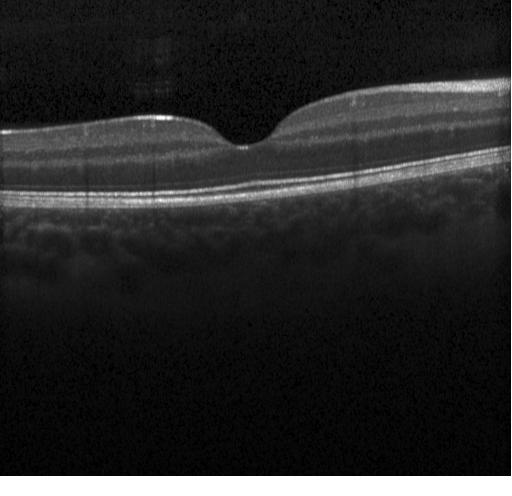 Optical coherence tomography B-scan. The scan shows no CNV, no DME, and no drusen.